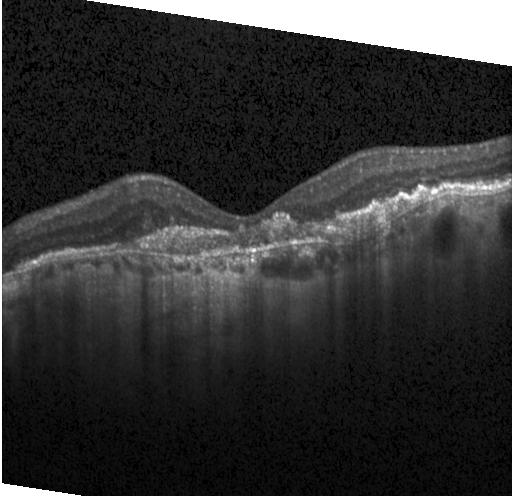
Macular OCT: choroidal neovascularization.